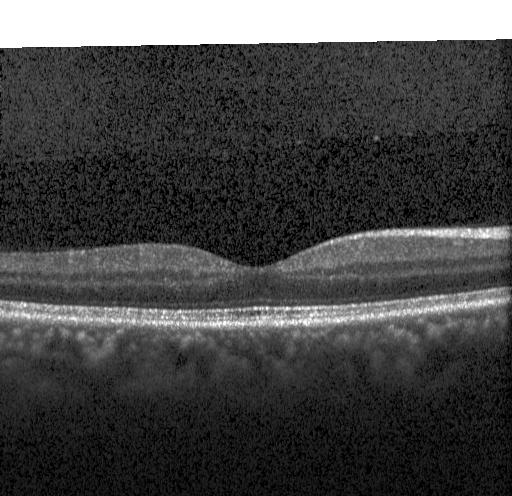
This B-scan demonstrates no choroidal neovascularization, diabetic macular edema, or drusen.